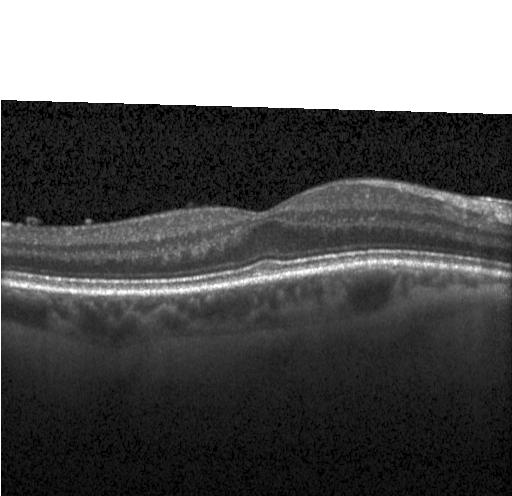

OCT line scan. Instrument: Heidelberg Spectralis
Diagnosis: no choroidal neovascularization, no diabetic macular edema, and no drusen.